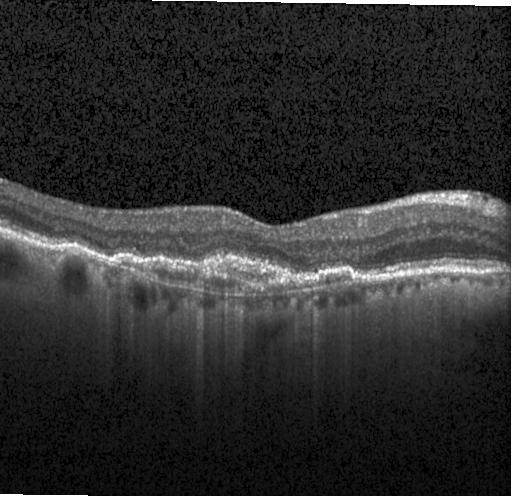

Heidelberg Spectralis OCT system. OCT B-scan. Spectral-domain OCT
Impression: choroidal neovascularization.